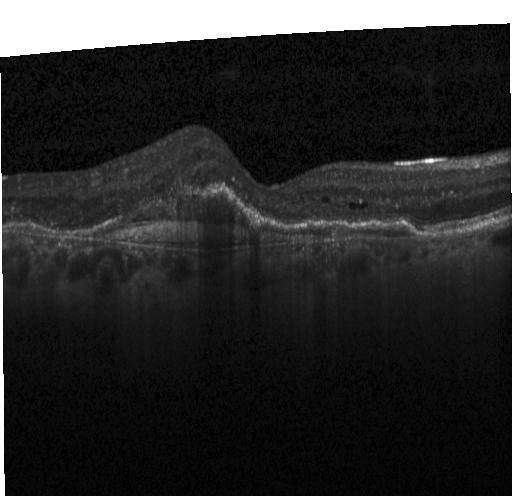

OCT line scan; instrument: Heidelberg Spectralis. Assessment: choroidal neovascularization (CNV).